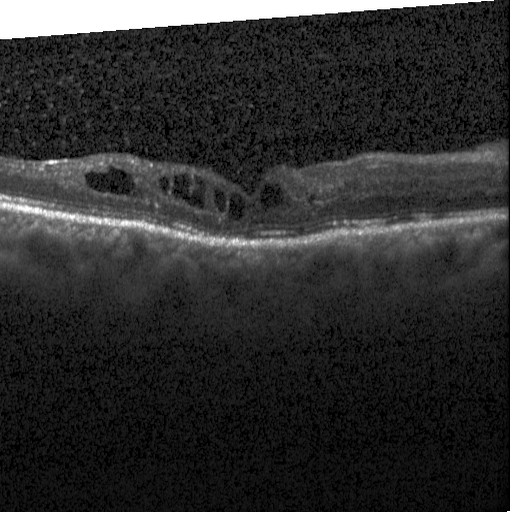
Dx: diabetic macular edema (DME).